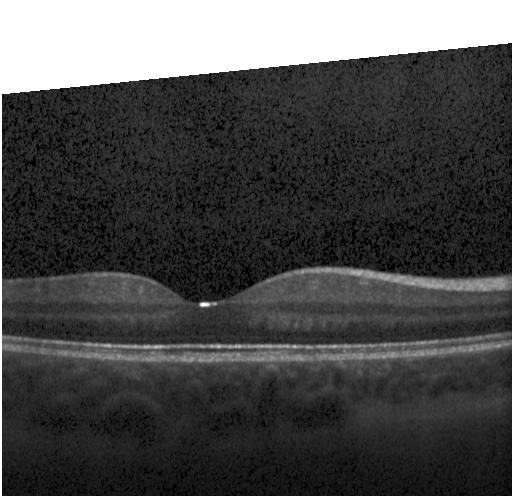
OCT finding: no choroidal neovascularization, no diabetic macular edema, and no drusen.